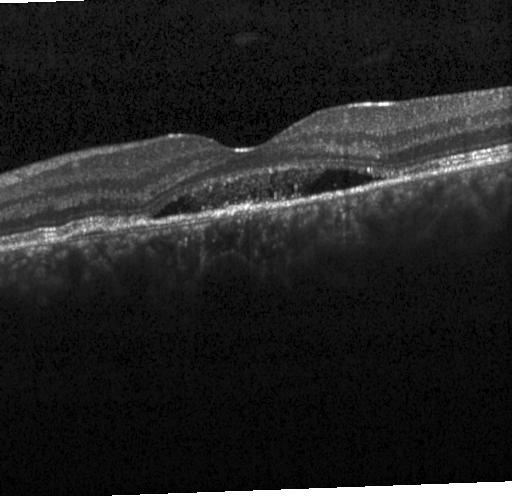

Acquired on a Heidelberg Spectralis, SD-OCT, centered on the fovea, optical coherence tomography B-scan.
A choroidal neovascular membrane.